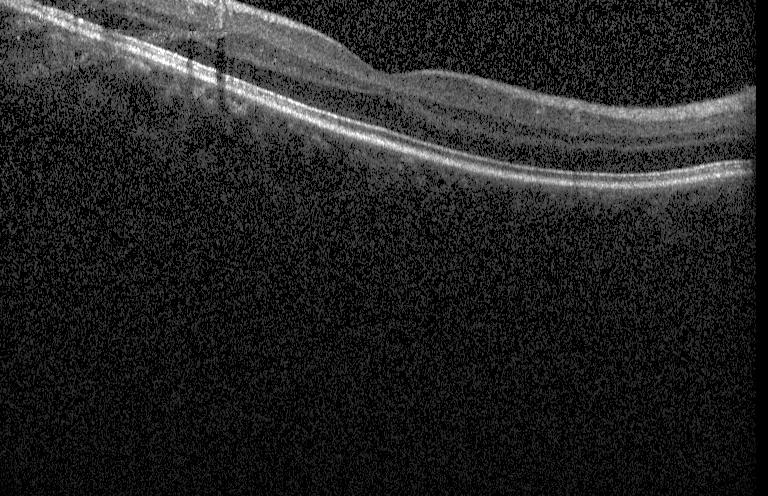
Acquired on a Heidelberg Spectralis, optical coherence tomography scan.
Impression: no choroidal neovascularization, no diabetic macular edema, and no drusen.